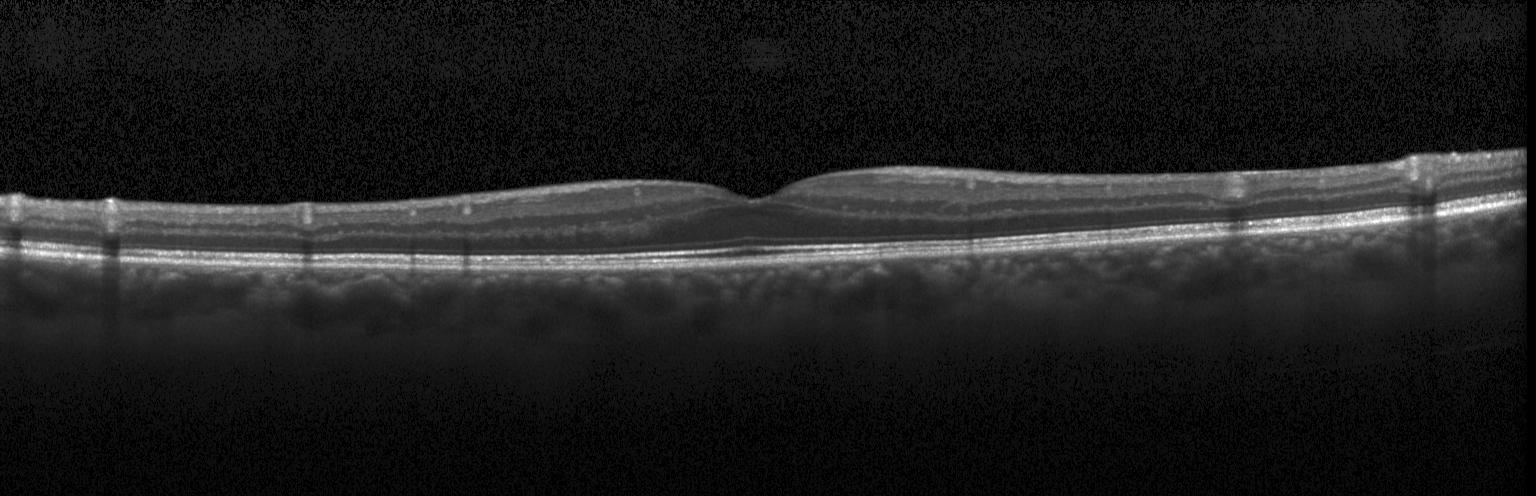
Optical coherence tomography B-scan.
Impression: neither choroidal neovascularization, diabetic macular edema, nor drusen.